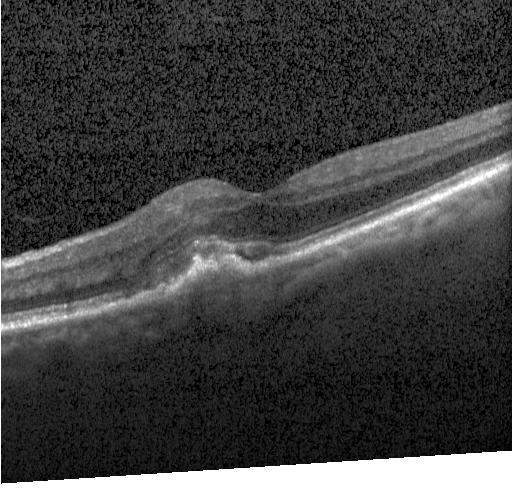

Retinal OCT cross-section — OCT finding: a choroidal neovascular membrane.